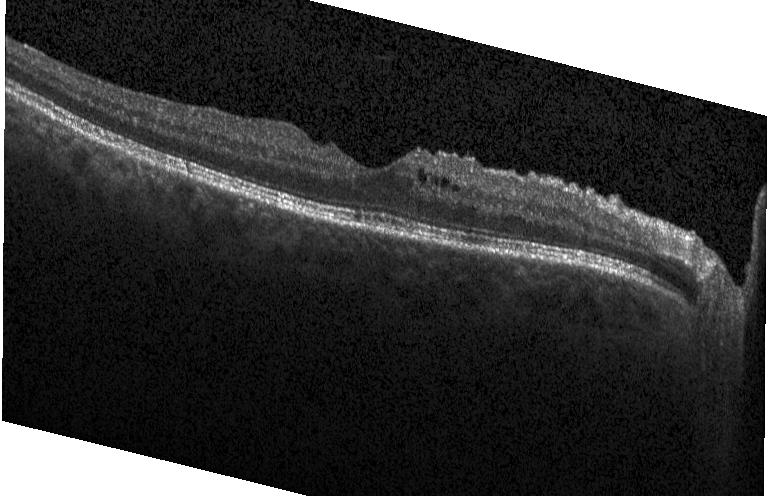 Retinal OCT cross-section.
OCT finding: diabetic macular edema (DME).